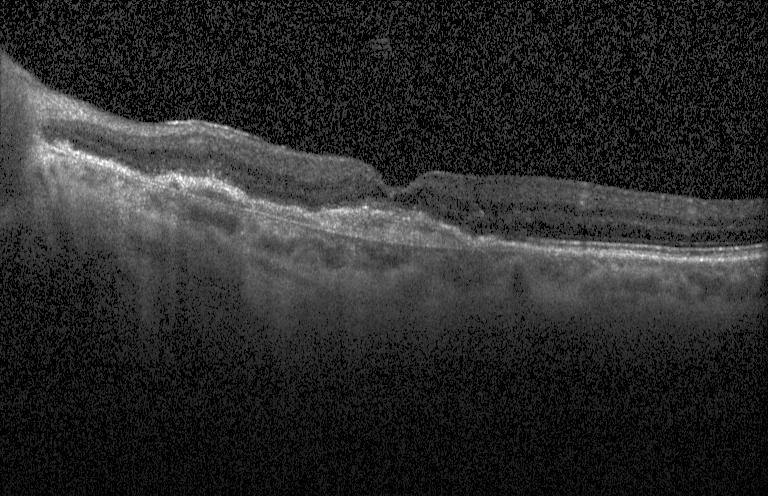 OCT B-scan
Finding: CNV.